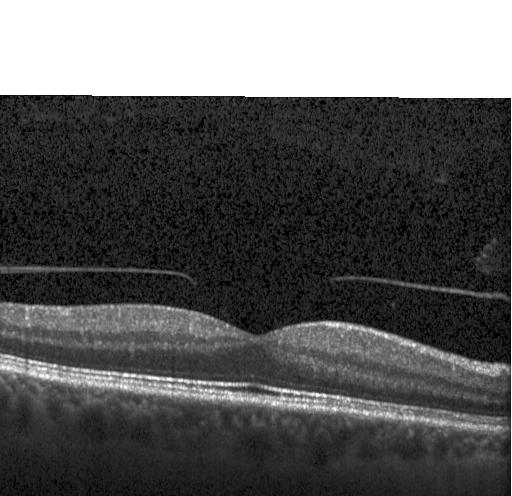

Acquired on a Heidelberg Spectralis; centered on the fovea; retinal OCT B-scan
Diagnosis: no evidence of choroidal neovascularization, diabetic macular edema, or drusen.